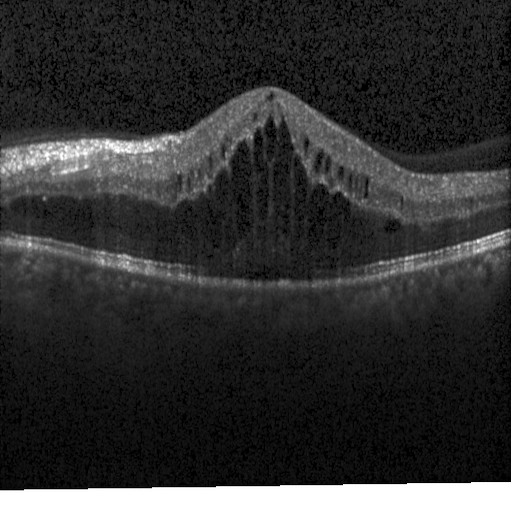

Acquired on a Heidelberg Spectralis, spectral-domain OCT, OCT line scan, fovea-centered.
Finding: diabetic macular edema.